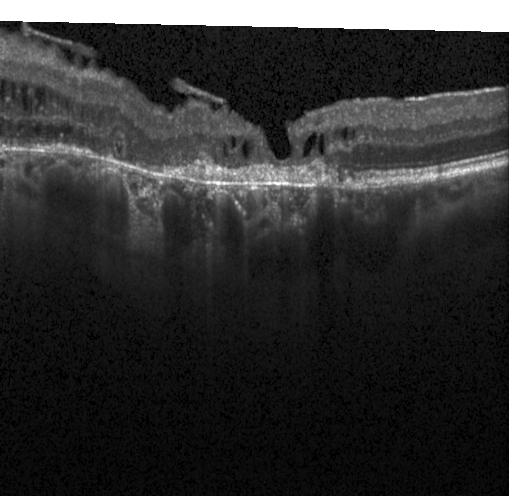 OCT line scan
Impression: a choroidal neovascular membrane.